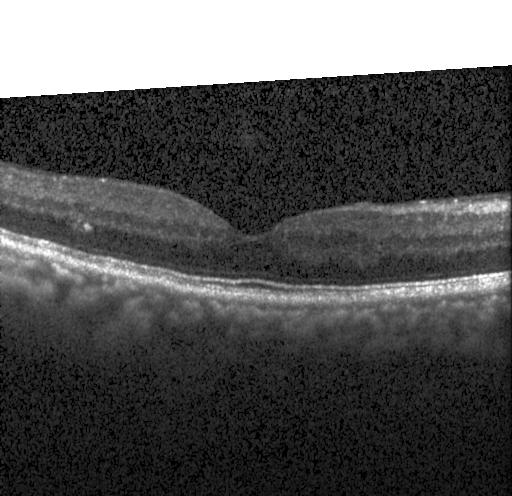
Fovea-centered · acquired on a Heidelberg Spectralis · spectral-domain OCT · retinal OCT B-scan.
OCT finding: no CNV, DME, or drusen.